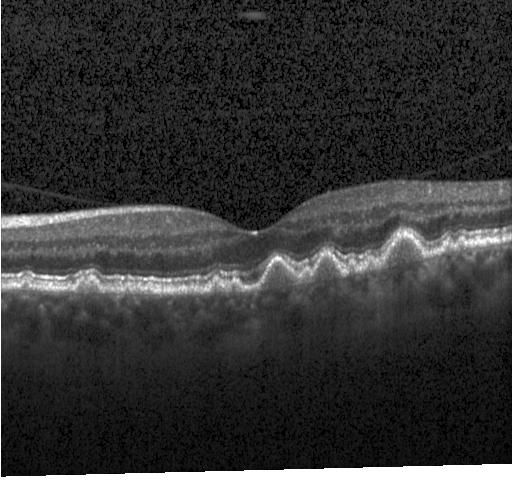
Spectral-domain OCT B-scan: sub-RPE drusenoid deposits.